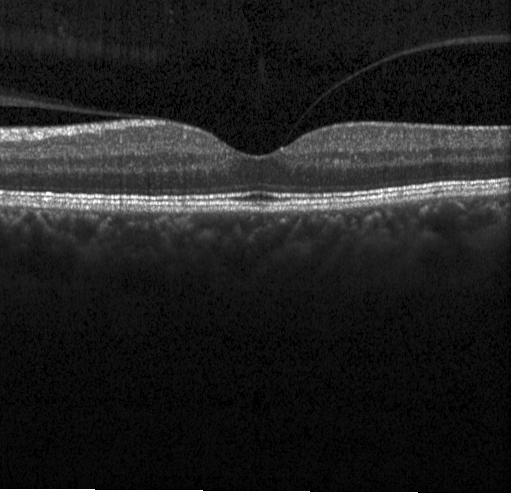
Horizontal scan through the fovea; optical coherence tomography scan; Heidelberg Spectralis OCT system; spectral-domain optical coherence tomography.
Impression: no choroidal neovascularization, diabetic macular edema, or drusen.